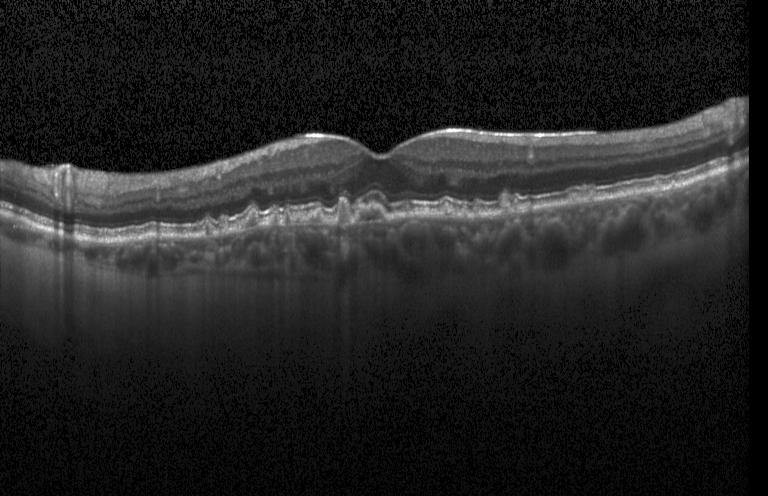

OCT B-scan
Impression: multiple drusen.